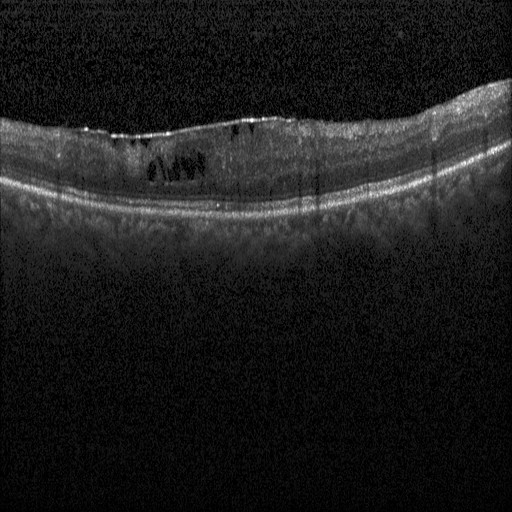
Through the macula, optical coherence tomography scan.
Diagnosis: DME.